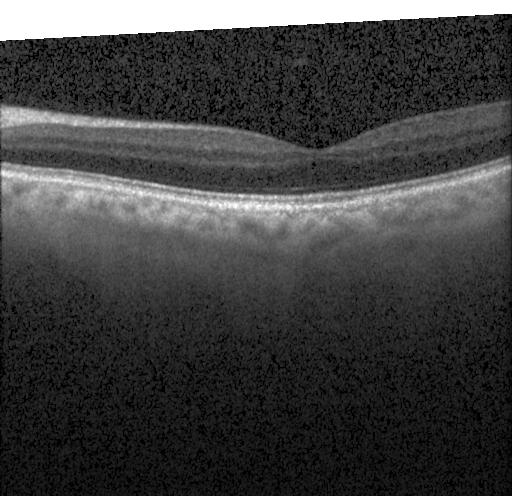 OCT scan showing no evidence of choroidal neovascularization, diabetic macular edema, or drusen.